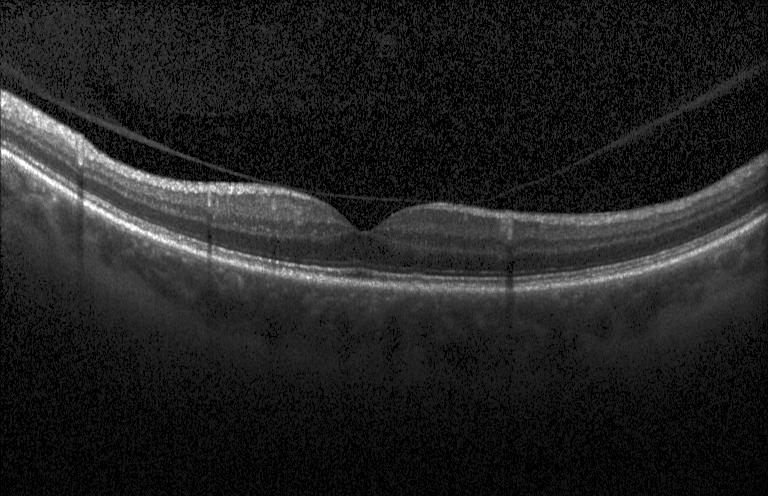 Centered on the fovea. Spectral-domain OCT. Instrument: Heidelberg Spectralis. Optical coherence tomography scan. Dx: no choroidal neovascularization, diabetic macular edema, or drusen.